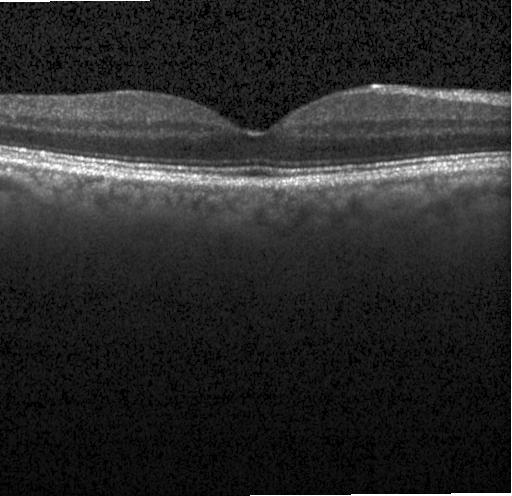
Spectral-domain optical coherence tomography · fovea-centered · retinal OCT cross-section · Heidelberg Spectralis OCT system. Assessment: no choroidal neovascularization, no diabetic macular edema, and no drusen.